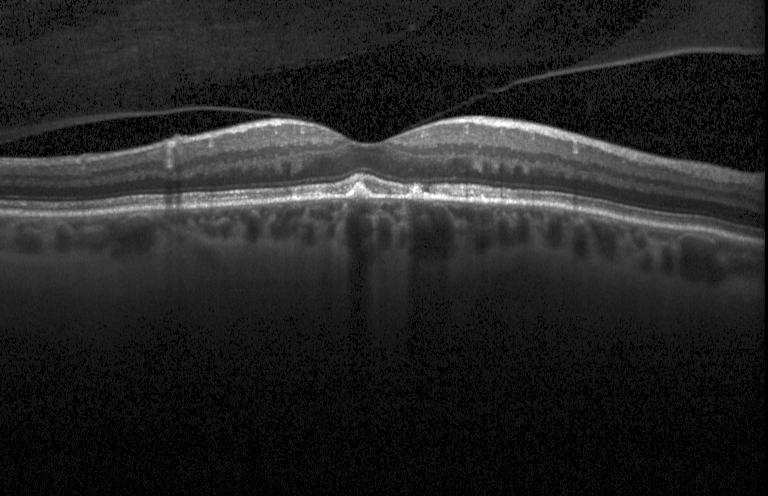

Heidelberg Spectralis; spectral-domain optical coherence tomography; optical coherence tomography B-scan — Finding: sub-RPE drusenoid deposits.